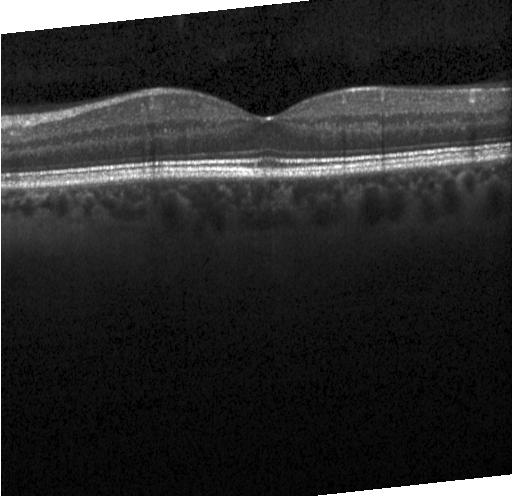
Spectral-domain optical coherence tomography; centered on the fovea; retinal OCT cross-section; instrument: Heidelberg Spectralis
Diagnosis: no evidence of choroidal neovascularization, diabetic macular edema, or drusen.